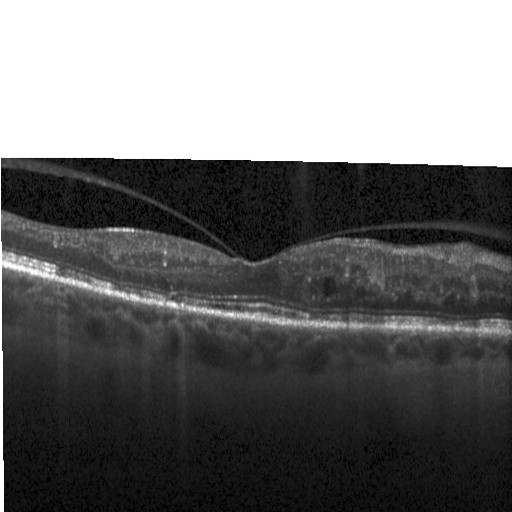
Retinal OCT cross-section. Through the macula. Instrument: Heidelberg Spectralis. Spectral-domain optical coherence tomography
Diagnosis: diabetic macular edema.